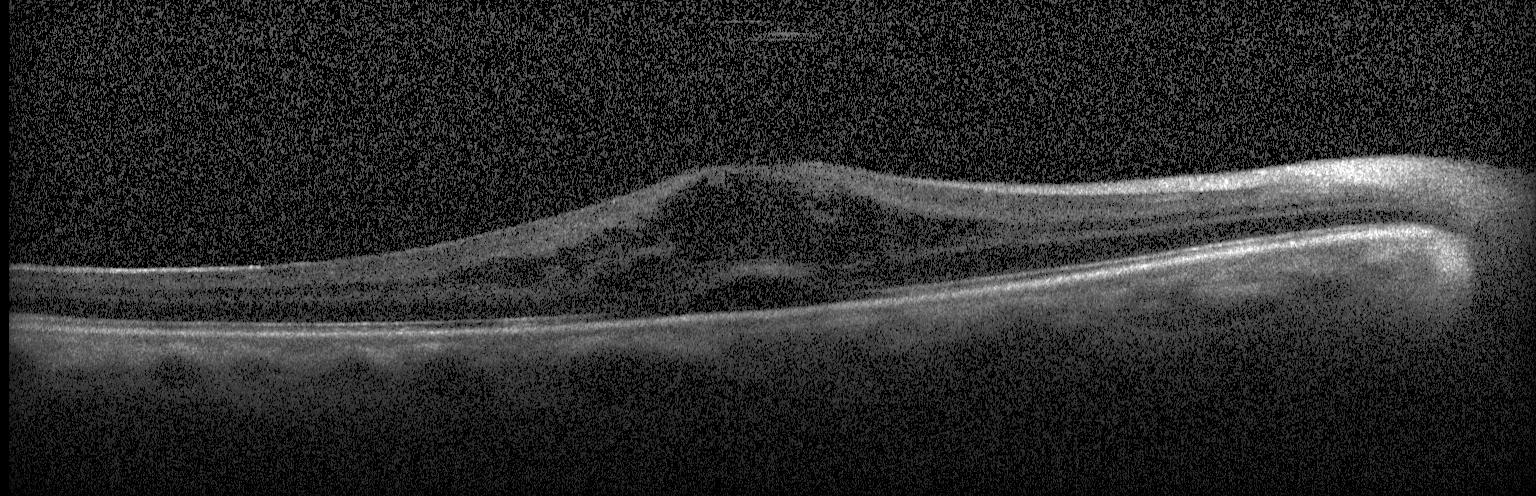

Retinal OCT cross-section. Horizontal scan through the fovea.
Impression: DME.